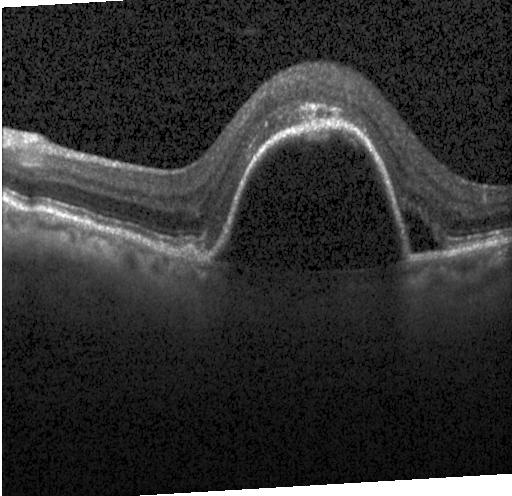
Optical coherence tomography B-scan.
The scan shows choroidal neovascularization (CNV).